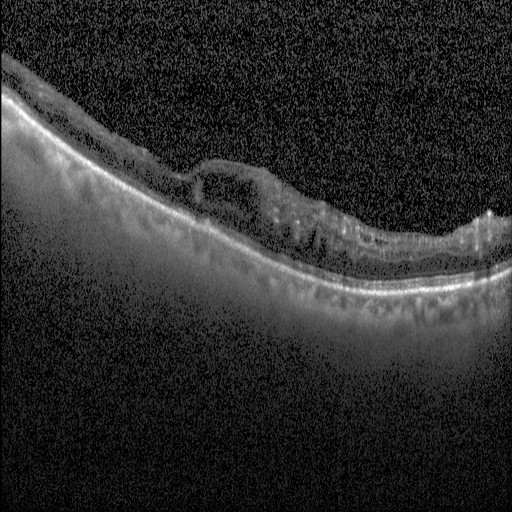 OCT scan showing diabetic macular edema (DME).